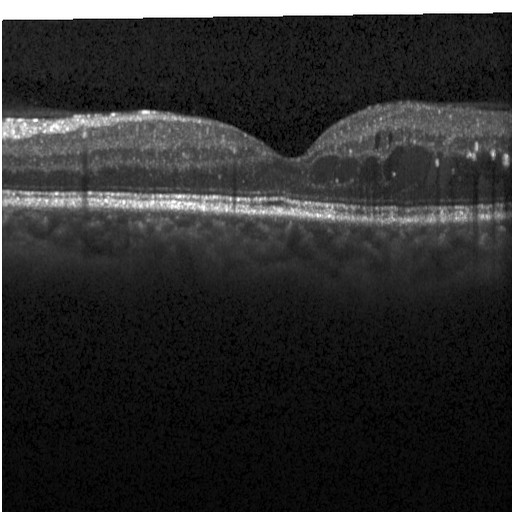
Macular scan. Heidelberg Spectralis. Retinal OCT cross-section. SD-OCT — Assessment: diabetic macular edema (DME).